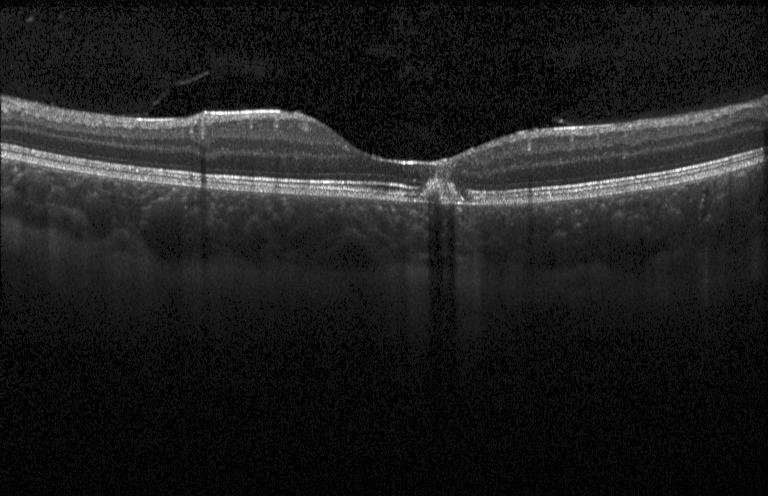

OCT line scan.
Impression: choroidal neovascularization.